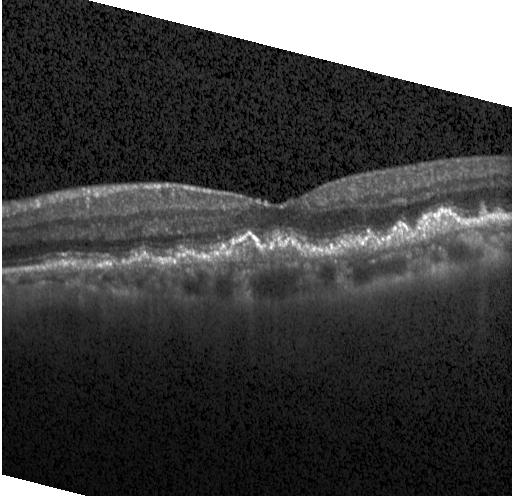

Impression: choroidal neovascularization (CNV).